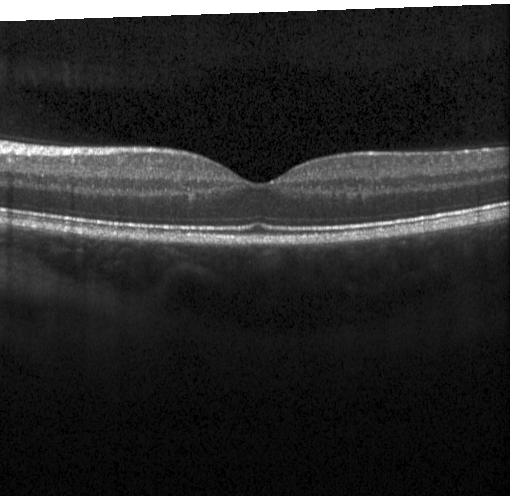

The scan shows neither CNV, DME, nor drusen.